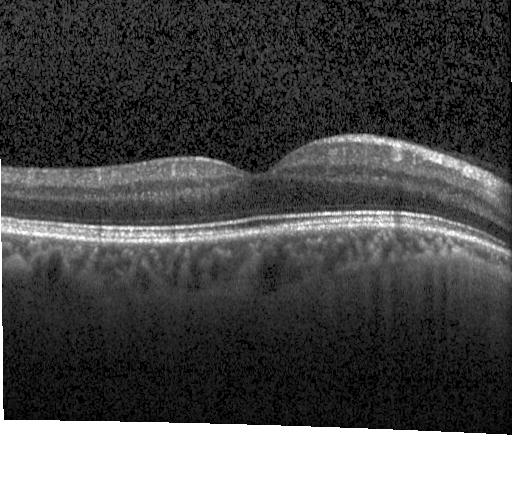 OCT finding: no CNV, DME, or drusen.